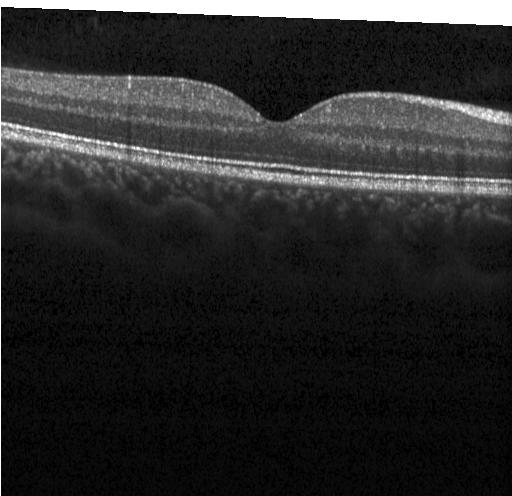

Finding: no choroidal neovascularization, diabetic macular edema, or drusen.